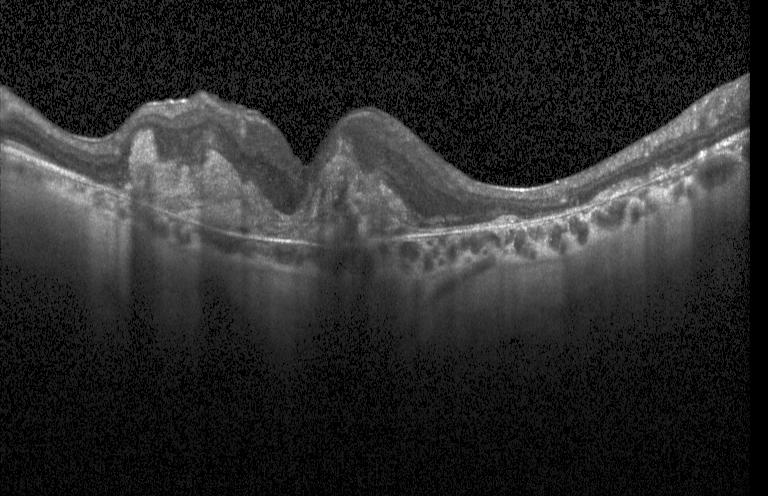 Assessment: CNV.